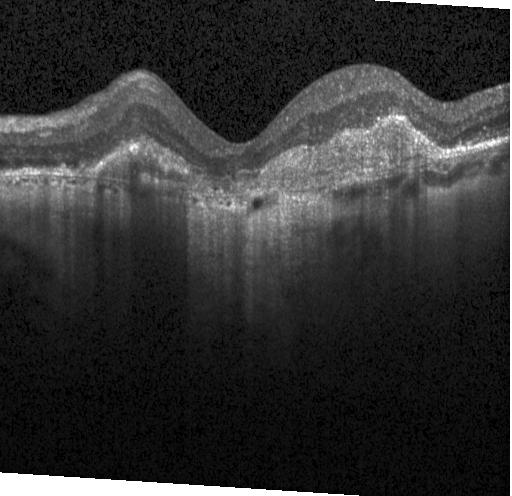 Optical coherence tomography scan, SD-OCT, fovea-centered — A choroidal neovascular membrane.